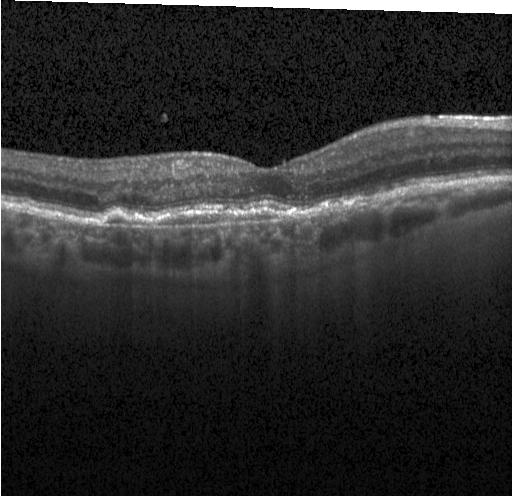
Assessment: a choroidal neovascular membrane.